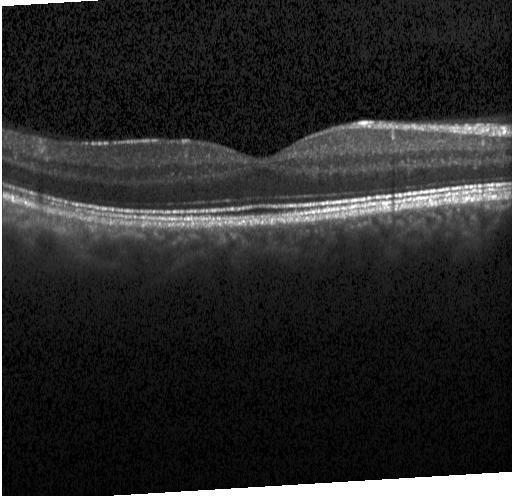 Spectral-domain OCT, centered on the fovea, Heidelberg Spectralis, optical coherence tomography scan.
Finding: no evidence of choroidal neovascularization, diabetic macular edema, or drusen.